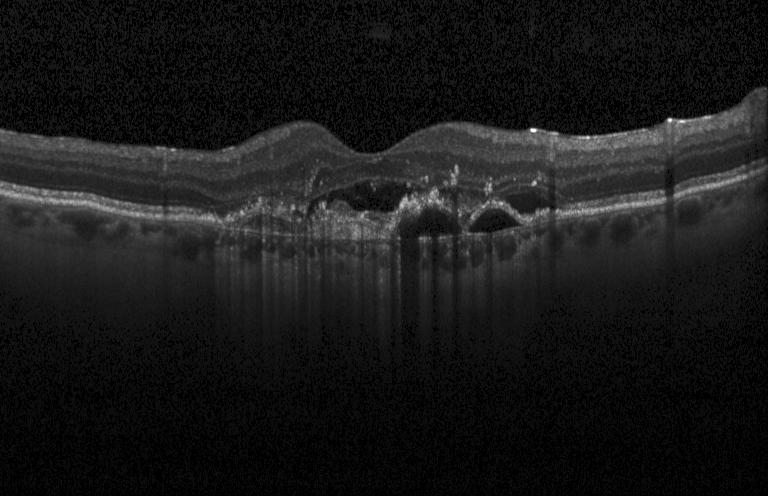 OCT finding: a choroidal neovascular membrane.